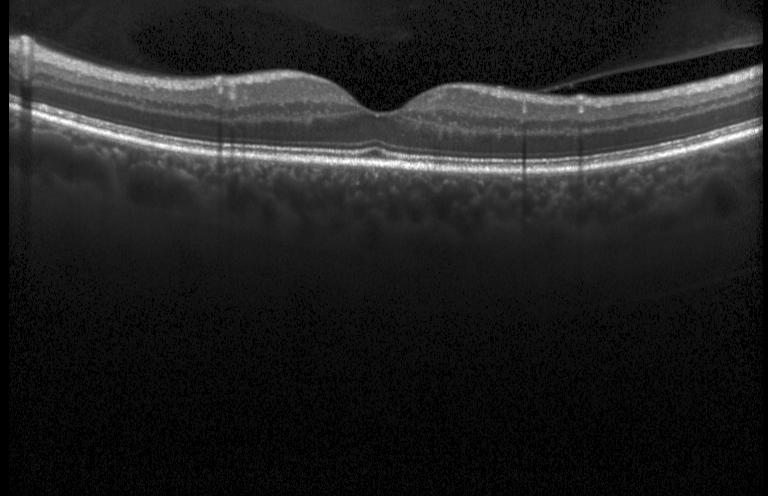

Dx: no evidence of choroidal neovascularization, diabetic macular edema, or drusen.